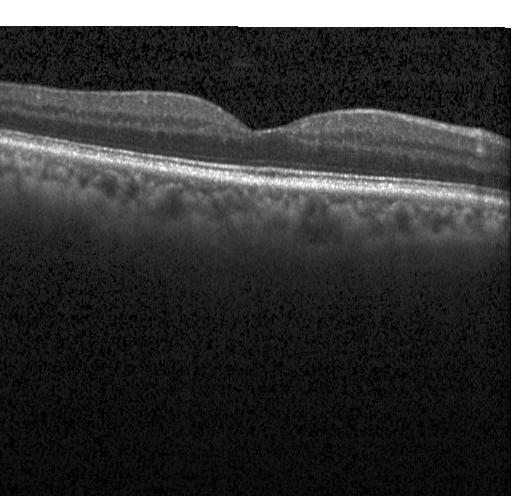
Fovea-centered, SD-OCT, retinal OCT cross-section — No CNV, DME, or drusen.